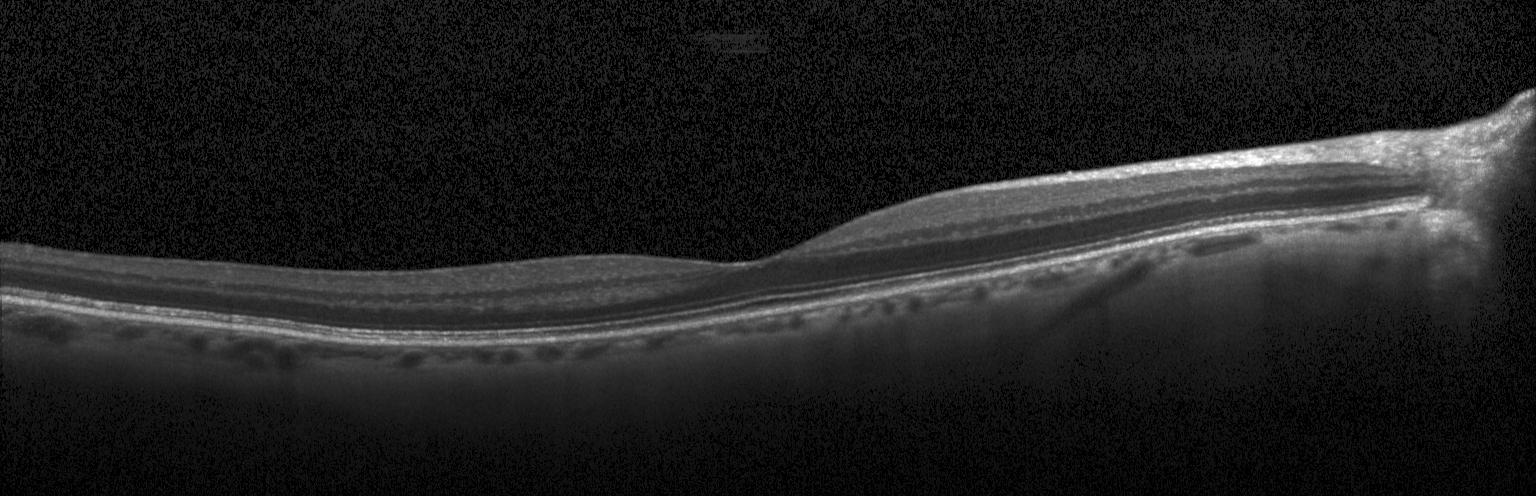
Optical coherence tomography scan
Diagnosis: no choroidal neovascularization, no diabetic macular edema, and no drusen.